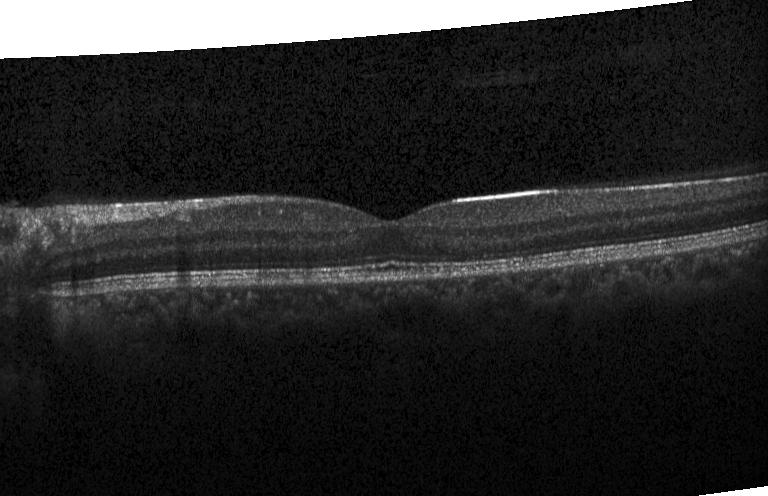

Optical coherence tomography scan.
Dx: neither choroidal neovascularization, diabetic macular edema, nor drusen.